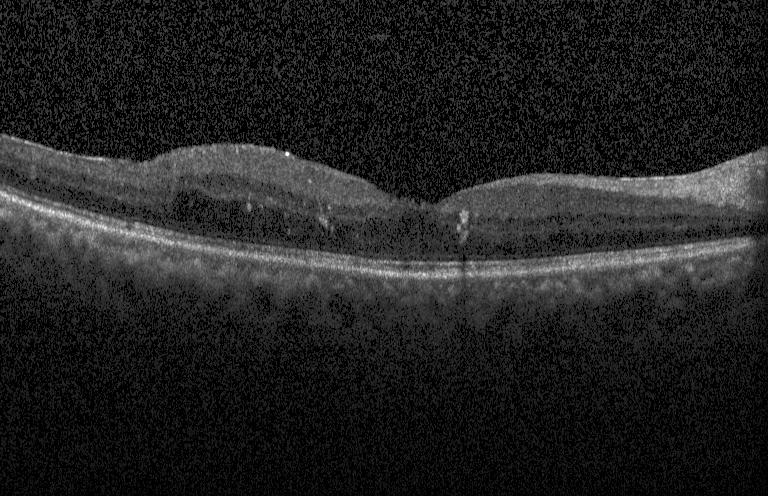

Optical coherence tomography B-scan — Assessment: DME.